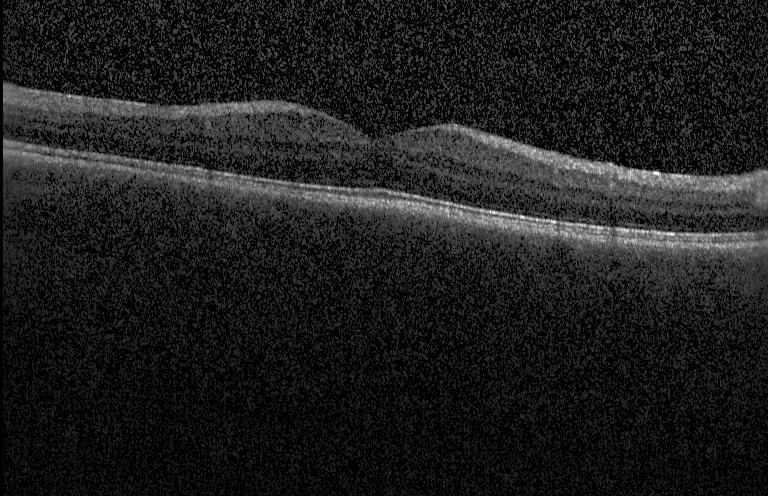 OCT scan showing no evidence of choroidal neovascularization, diabetic macular edema, or drusen.